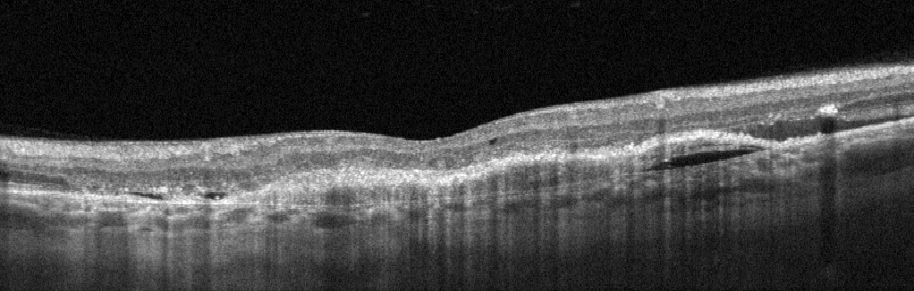 Optical coherence tomography scan. Right eye. Instrument: Optovue Avanti RTVue XR — Finding: age-related macular degeneration.